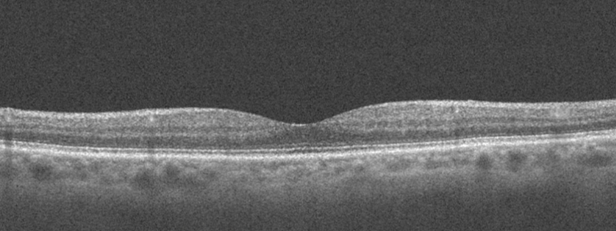 Retinal OCT cross-section — This B-scan demonstrates no evidence of AMD, DME, ERM, RAO, RVO, or VID.